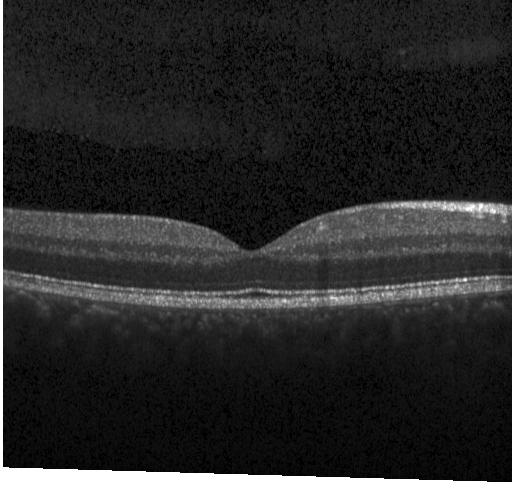

SD-OCT. Acquired on a Heidelberg Spectralis. OCT line scan.
The scan shows no choroidal neovascularization, diabetic macular edema, or drusen.